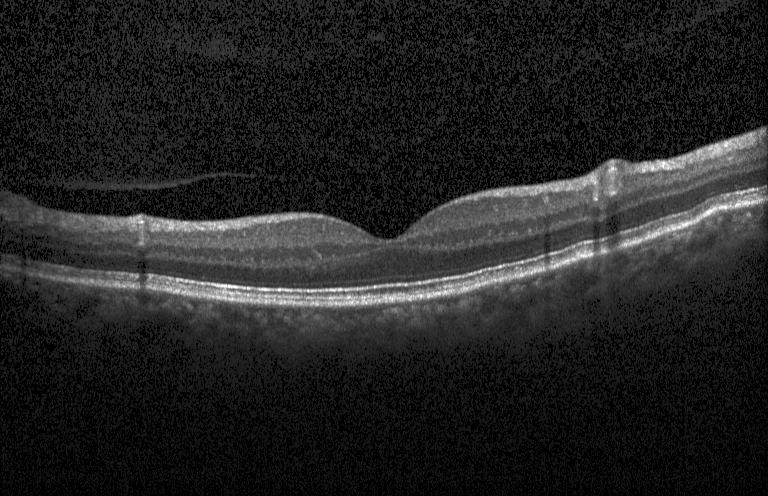 Fovea-centered. Optical coherence tomography scan
Impression: no choroidal neovascularization, diabetic macular edema, or drusen.